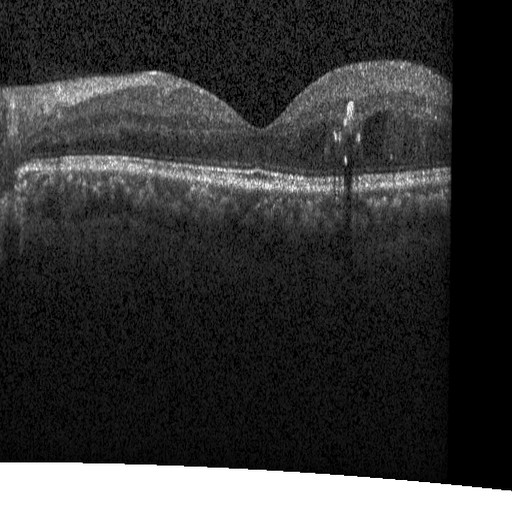

This B-scan demonstrates diabetic macular edema.